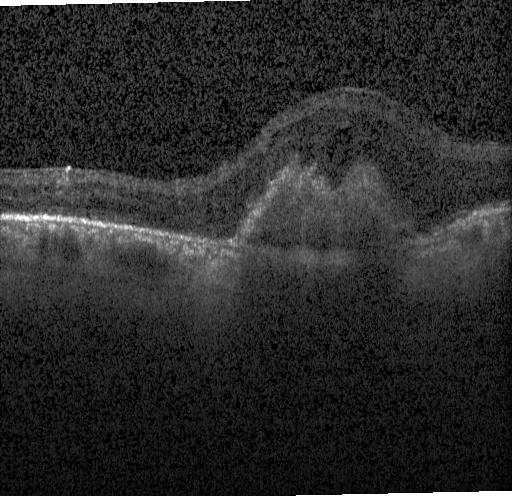

This B-scan demonstrates a choroidal neovascular membrane.